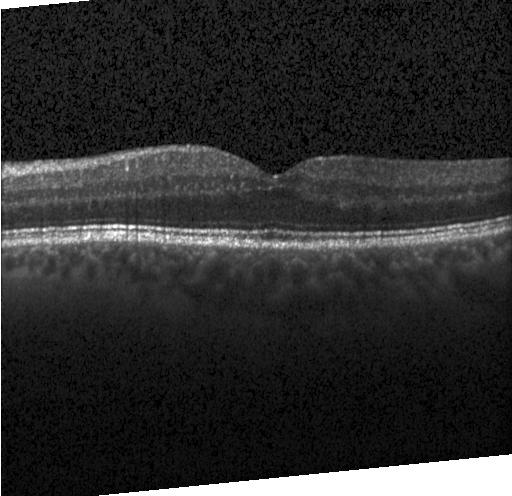

Spectral-domain OCT · acquired on a Heidelberg Spectralis · optical coherence tomography scan — Finding: no CNV, DME, or drusen.